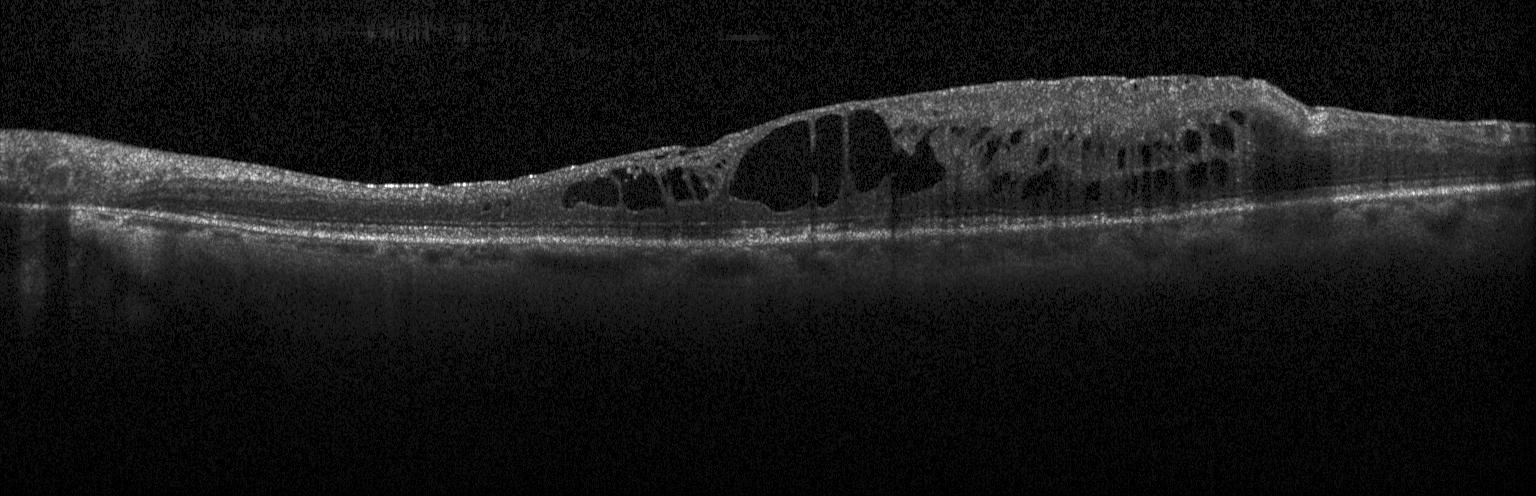
Centered on the fovea · spectral-domain OCT · Heidelberg Spectralis OCT system · retinal OCT cross-section. Impression: diabetic macular edema.